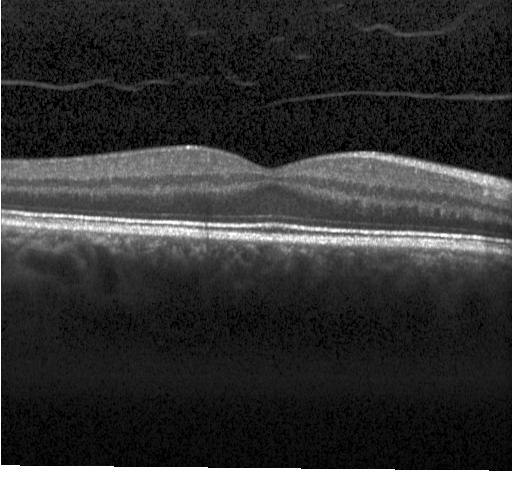
This B-scan demonstrates no evidence of choroidal neovascularization, diabetic macular edema, or drusen.